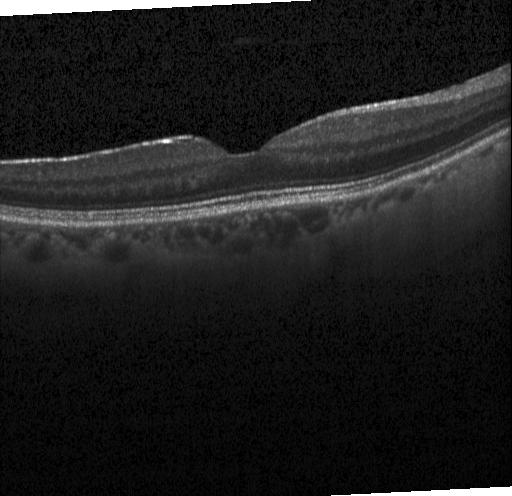

SD-OCT; Heidelberg Spectralis; macular scan; retinal OCT B-scan. No evidence of choroidal neovascularization, diabetic macular edema, or drusen.